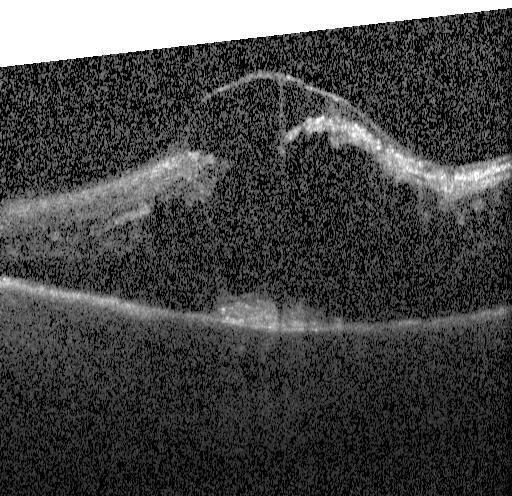
Optical coherence tomography scan. Macular scan — OCT finding: diabetic macular edema (DME).